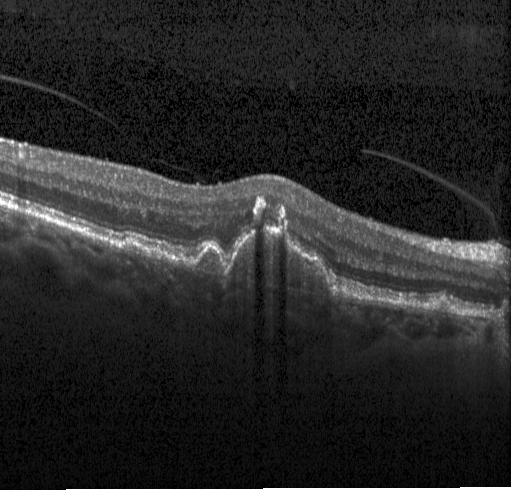 OCT finding: CNV.